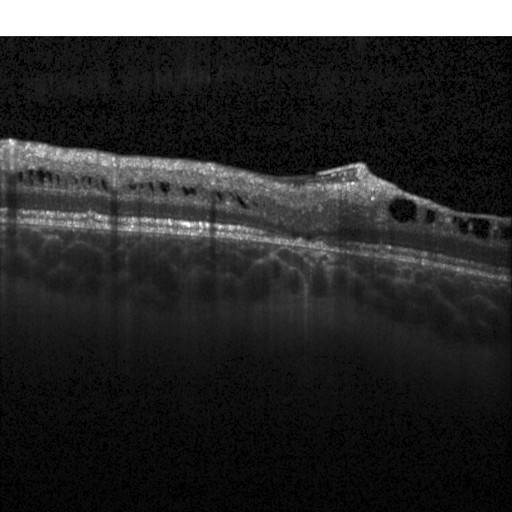
Assessment: DME.